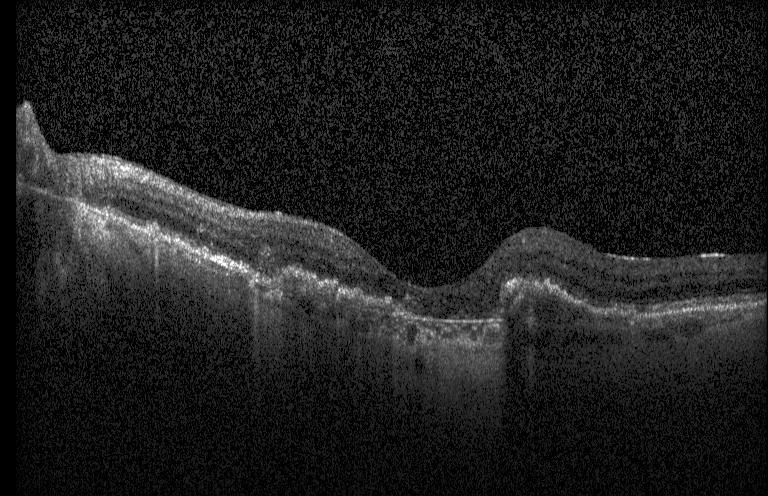
Optical coherence tomography scan. Finding: choroidal neovascularization.